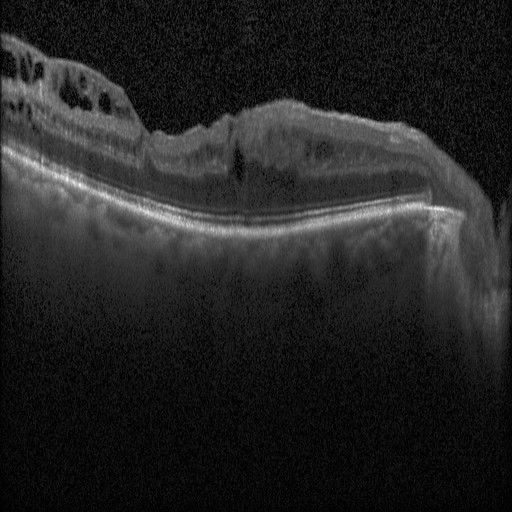
Spectral-domain optical coherence tomography; retinal OCT B-scan; centered on the fovea. Diagnosis: diabetic macular edema.